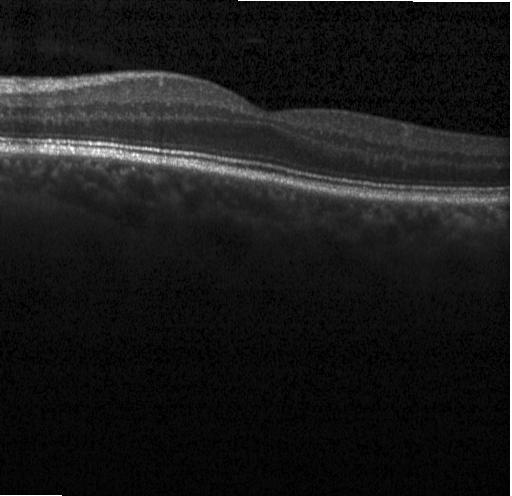

OCT B-scan showing no choroidal neovascularization, no diabetic macular edema, and no drusen.